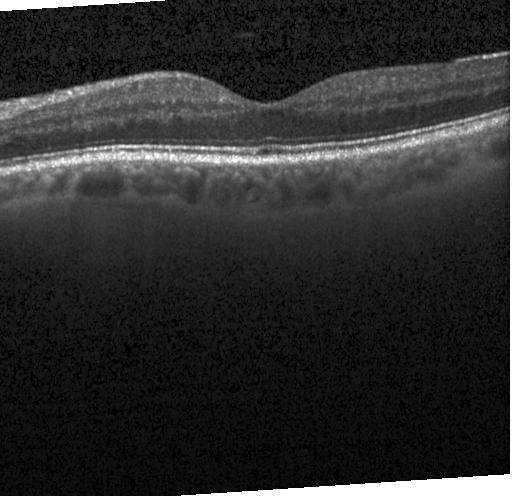 Retinal OCT B-scan, horizontal scan through the fovea, spectral-domain optical coherence tomography
Macular OCT: neither CNV, DME, nor drusen.